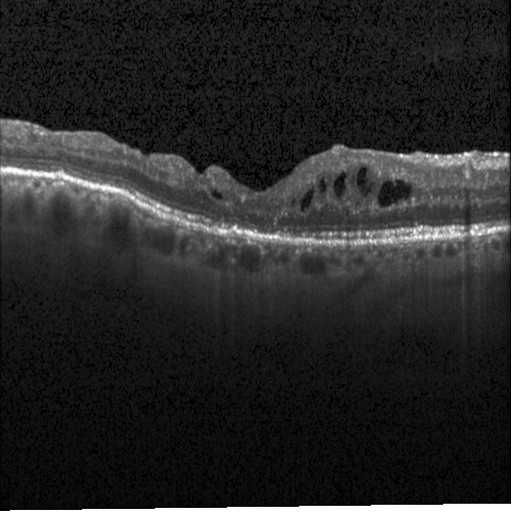

Diabetic macular edema.